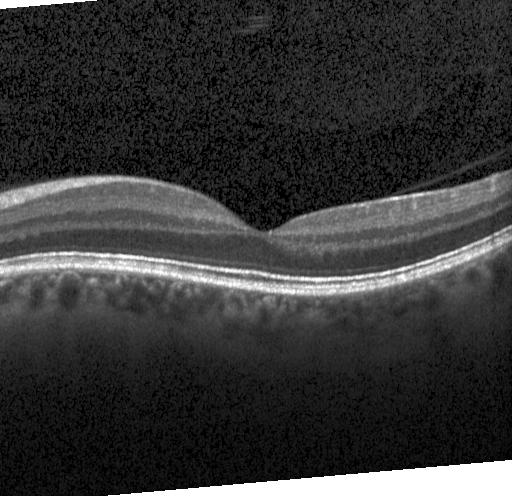

Spectral-domain OCT B-scan: no evidence of choroidal neovascularization, diabetic macular edema, or drusen.